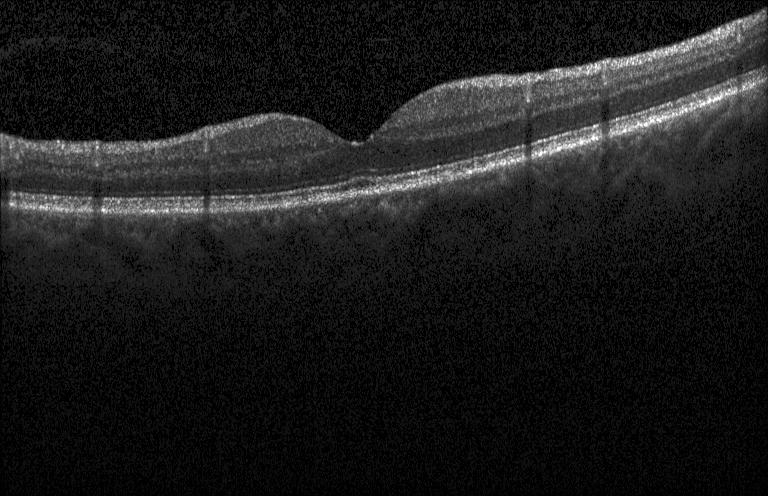

Retinal OCT B-scan. No evidence of choroidal neovascularization, diabetic macular edema, or drusen.